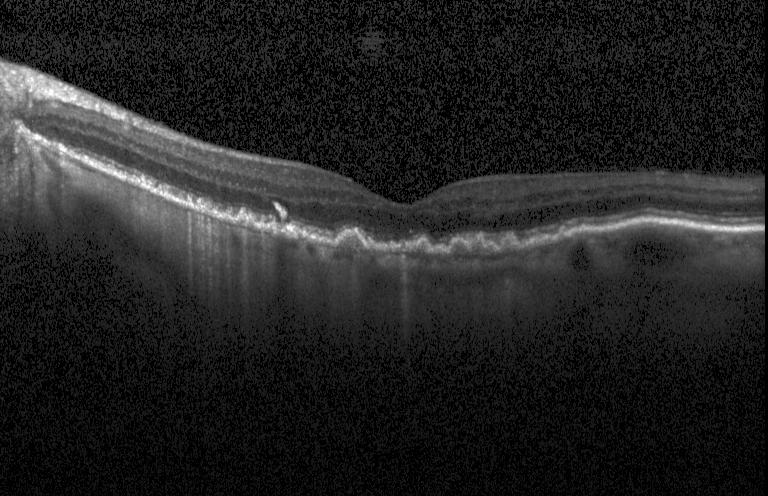 Retinal OCT B-scan · SD-OCT. Diagnosis: sub-RPE drusenoid deposits.